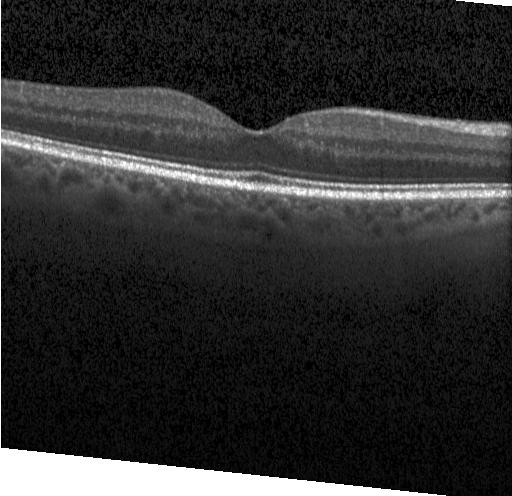

Instrument: Heidelberg Spectralis; spectral-domain optical coherence tomography; OCT line scan; centered on the fovea.
Diagnosis: no choroidal neovascularization, diabetic macular edema, or drusen.